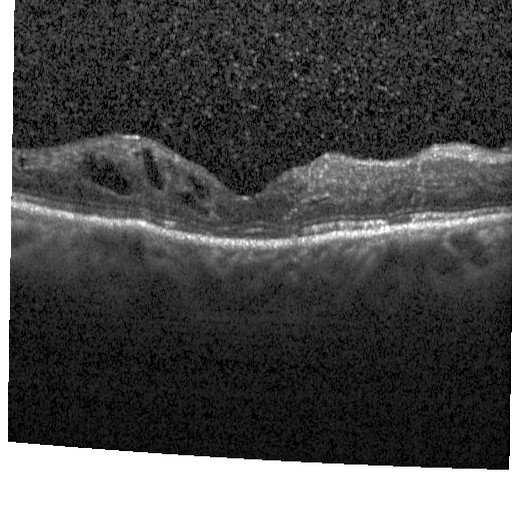
Spectral-domain OCT, retinal OCT cross-section. The scan shows DME.